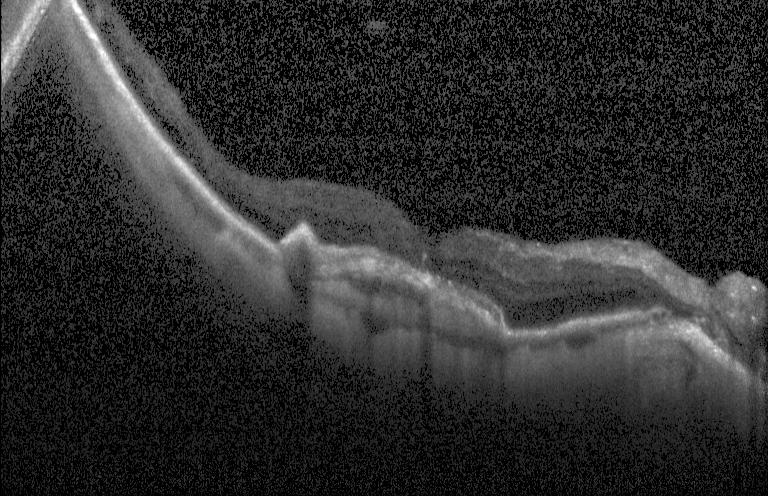 Retinal OCT cross-section — Finding: a choroidal neovascular membrane.